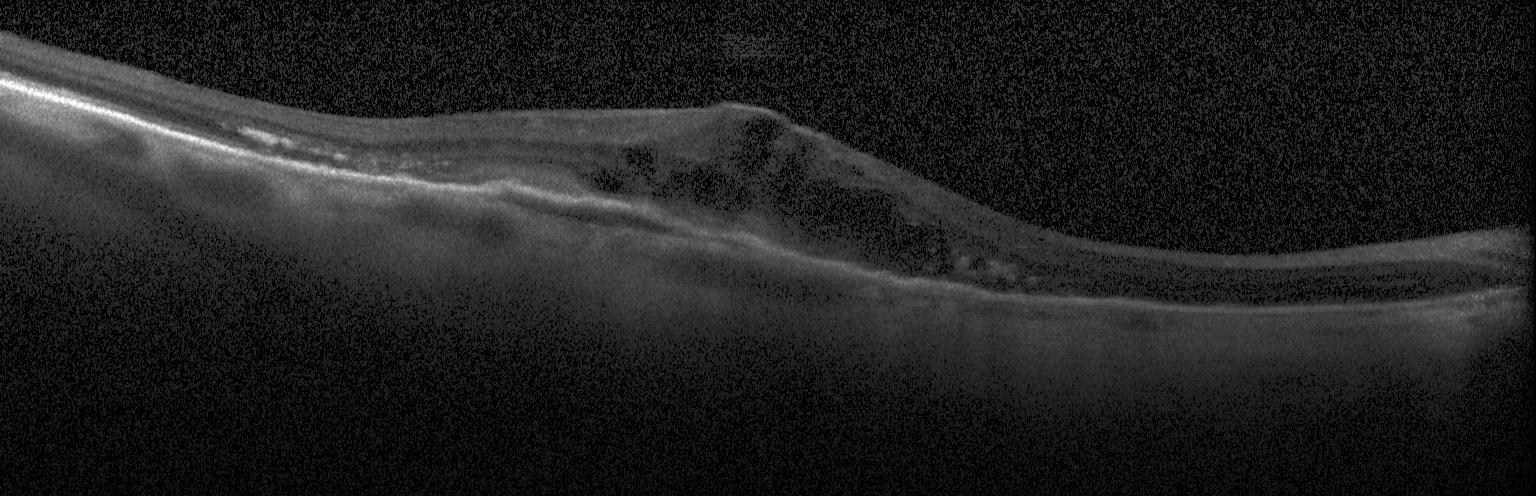
Finding: choroidal neovascularization.